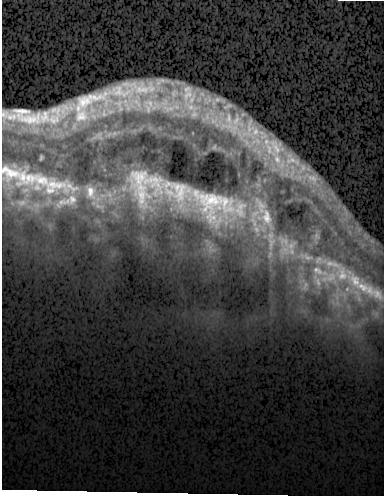 Horizontal scan through the fovea. Retinal OCT B-scan.
This B-scan demonstrates choroidal neovascularization.